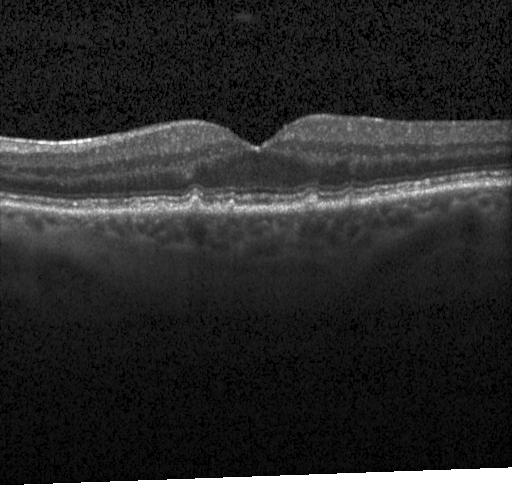

Spectral-domain OCT, horizontal scan through the fovea, retinal OCT cross-section, Heidelberg Spectralis.
Dx: multiple drusen.